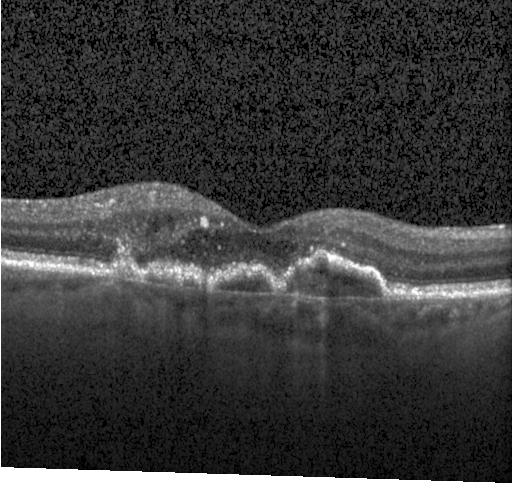 OCT B-scan · acquired on a Heidelberg Spectralis.
OCT finding: choroidal neovascularization (CNV).